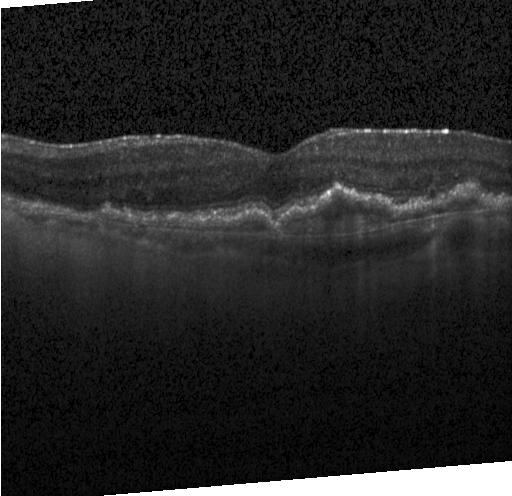 Finding: a choroidal neovascular membrane.